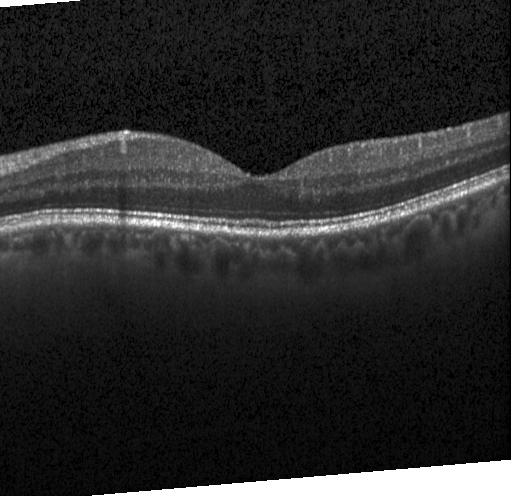 Assessment: neither choroidal neovascularization, diabetic macular edema, nor drusen.